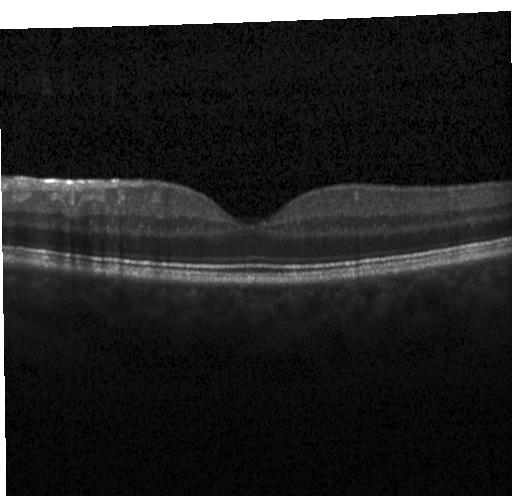
Macular scan; optical coherence tomography scan.
Impression: no evidence of choroidal neovascularization, diabetic macular edema, or drusen.